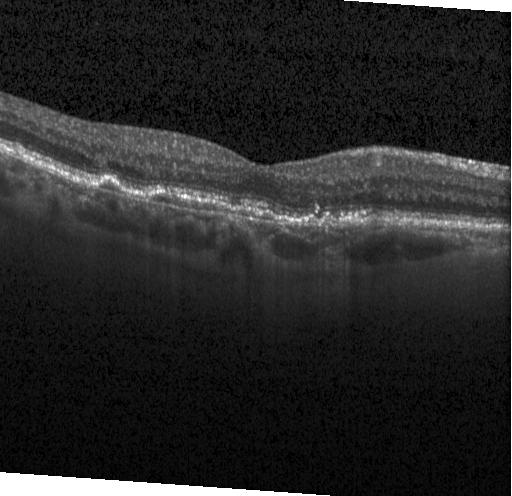

Finding: choroidal neovascularization (CNV).